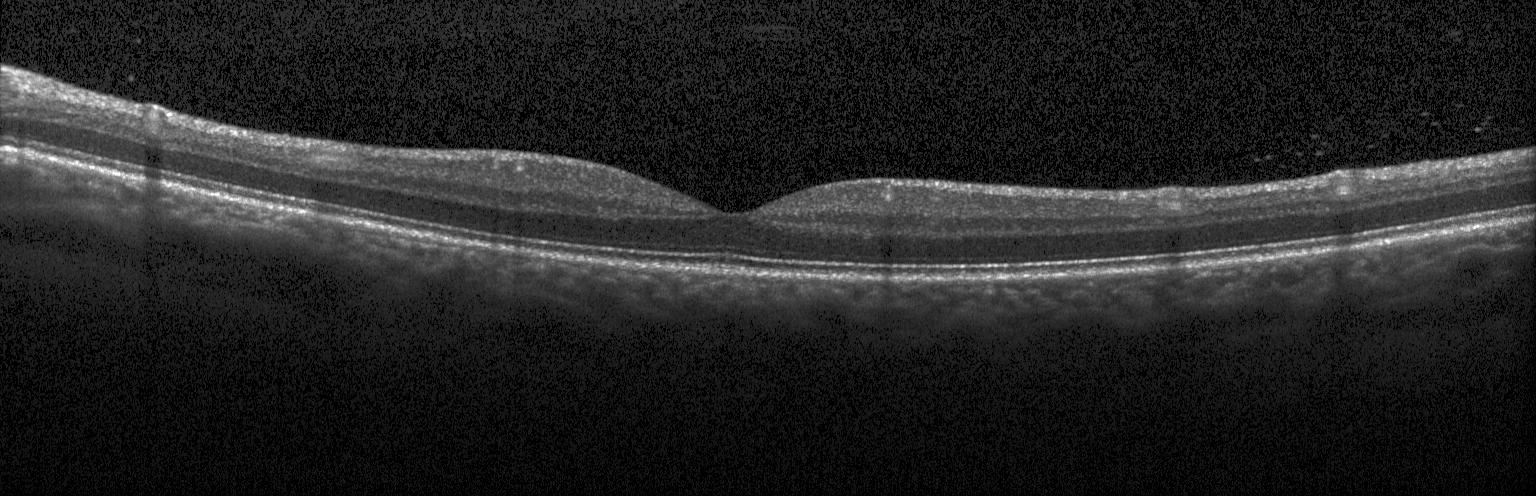

Spectral-domain OCT · Heidelberg Spectralis OCT system · OCT B-scan · centered on the fovea
Impression: no evidence of choroidal neovascularization, diabetic macular edema, or drusen.